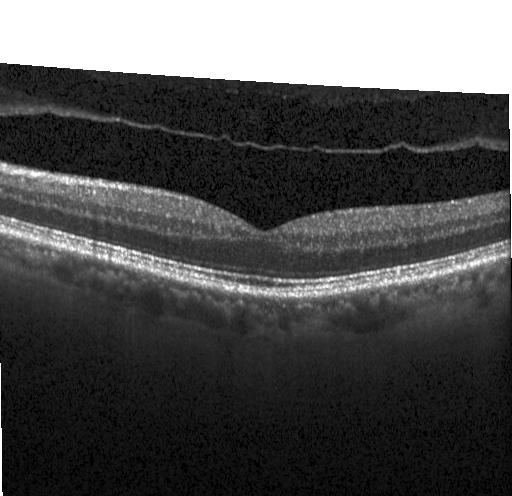
Optical coherence tomography scan
Assessment: neither choroidal neovascularization, diabetic macular edema, nor drusen.